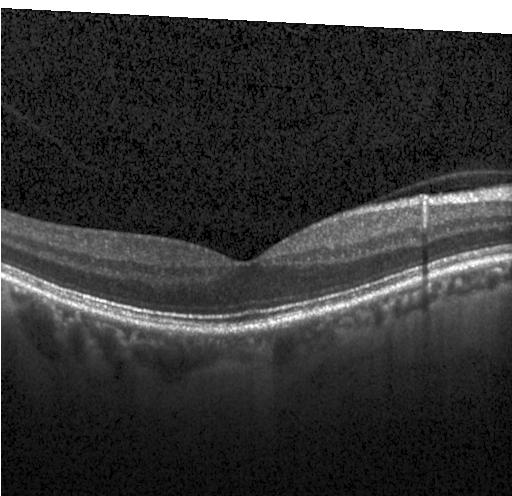
Optical coherence tomography B-scan — The scan shows no choroidal neovascularization, no diabetic macular edema, and no drusen.